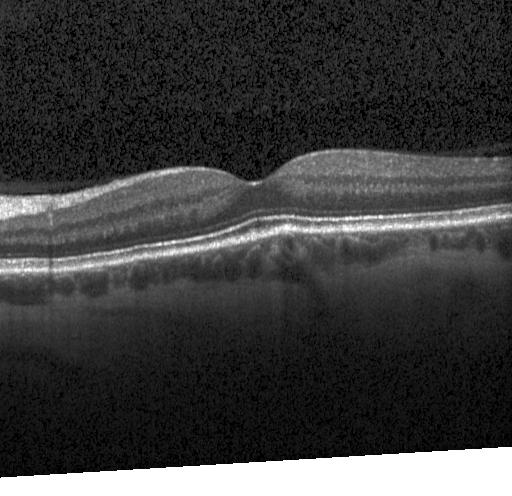
Acquired on a Heidelberg Spectralis; through the macula; optical coherence tomography scan; spectral-domain OCT
Diagnosis: no evidence of choroidal neovascularization, diabetic macular edema, or drusen.